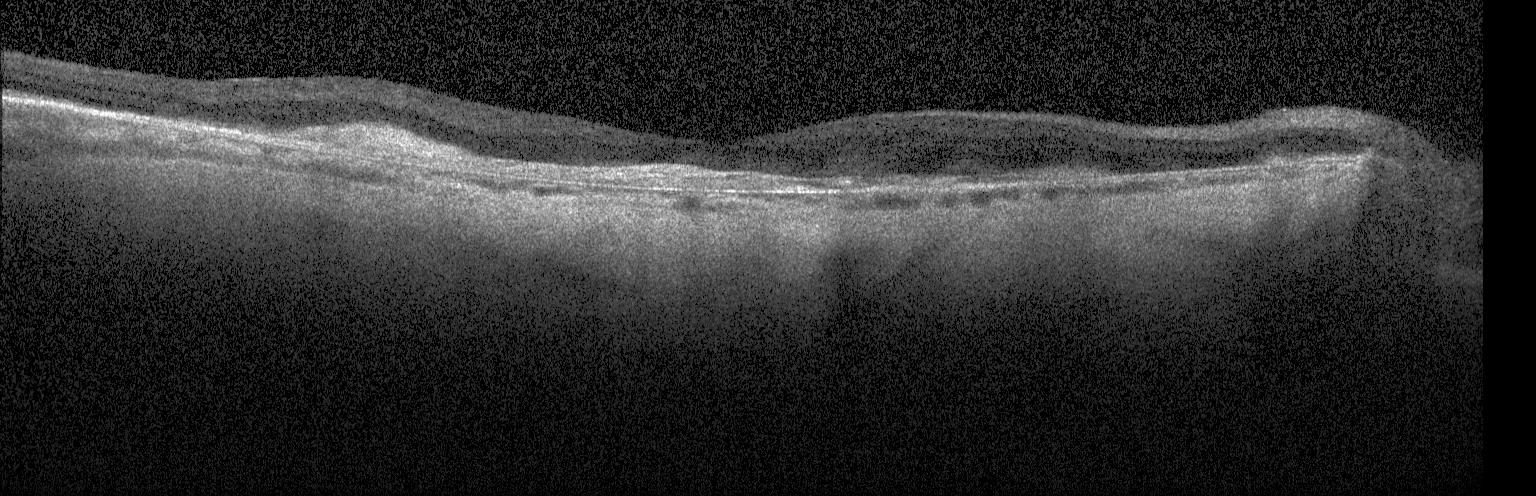
Impression: choroidal neovascularization.